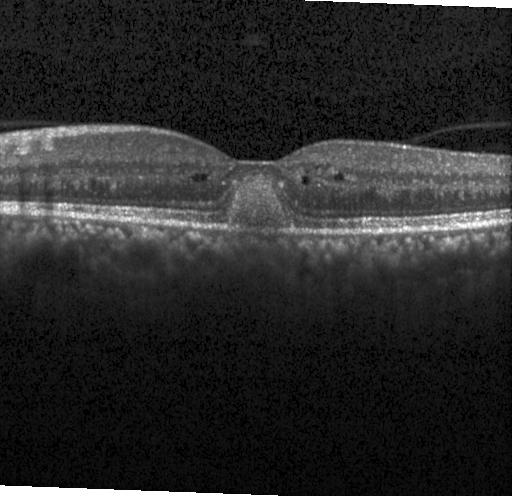
OCT B-scan. Fovea-centered. Spectral-domain optical coherence tomography. Instrument: Heidelberg Spectralis — Impression: a choroidal neovascular membrane.